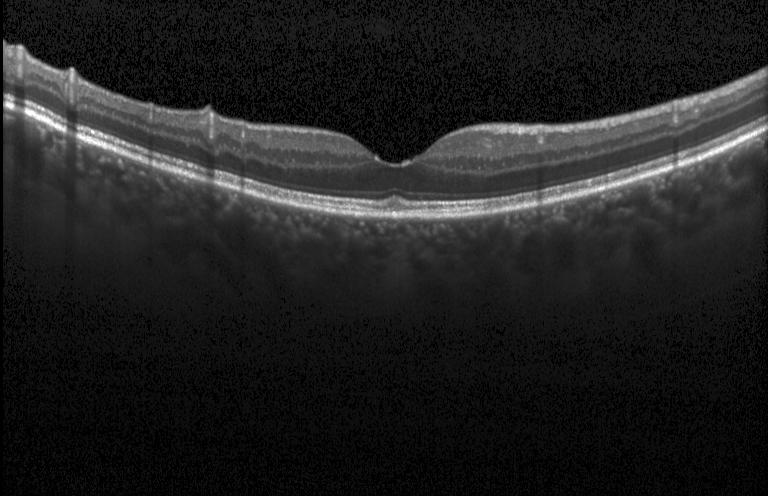

Heidelberg Spectralis · optical coherence tomography scan
Assessment: neither CNV, DME, nor drusen.